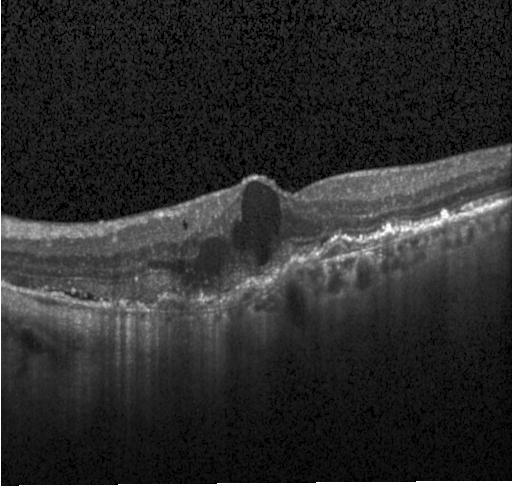

Impression: choroidal neovascularization (CNV).